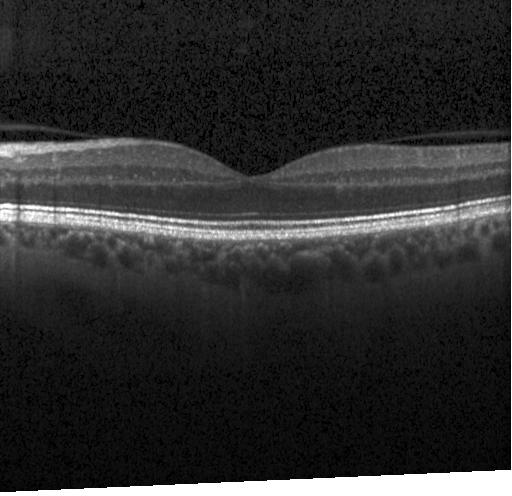
Retinal OCT cross-section — Dx: neither choroidal neovascularization, diabetic macular edema, nor drusen.